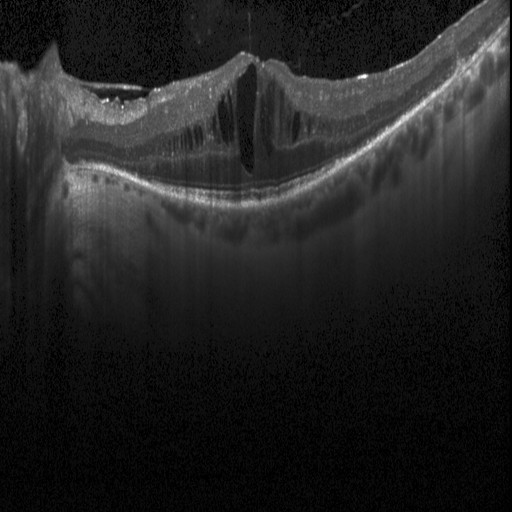

Centered on the fovea. OCT line scan
Impression: diabetic macular edema.